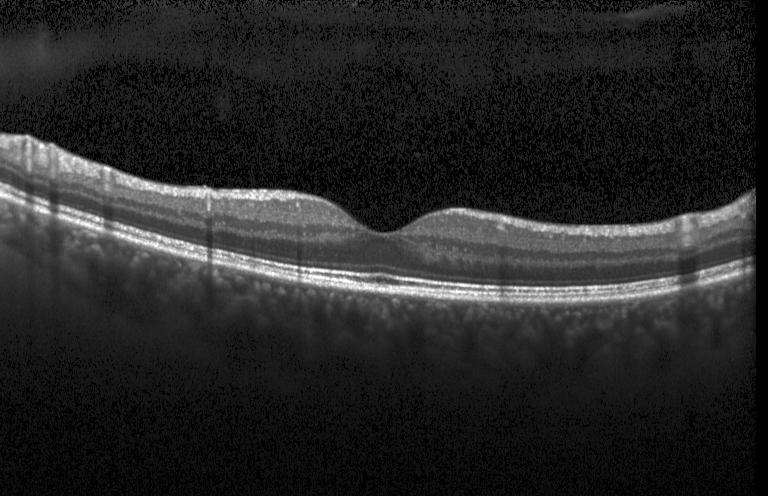

Optical coherence tomography B-scan; macular scan; spectral-domain optical coherence tomography; Heidelberg Spectralis — This B-scan demonstrates no CNV, DME, or drusen.